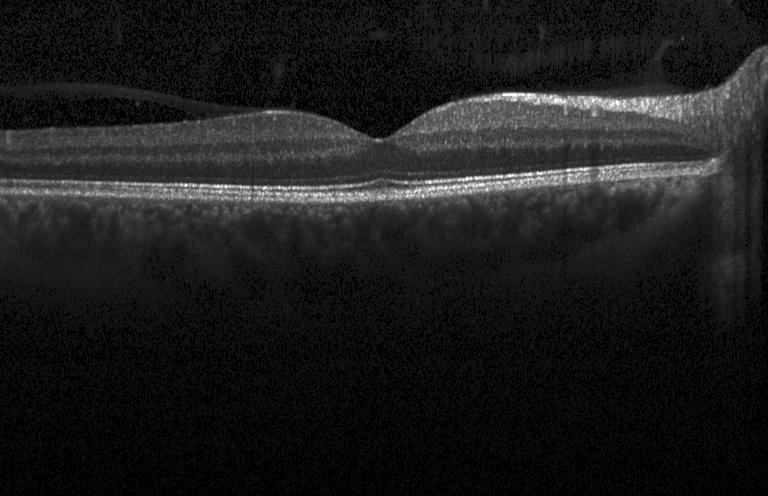
OCT finding: no evidence of choroidal neovascularization, diabetic macular edema, or drusen.